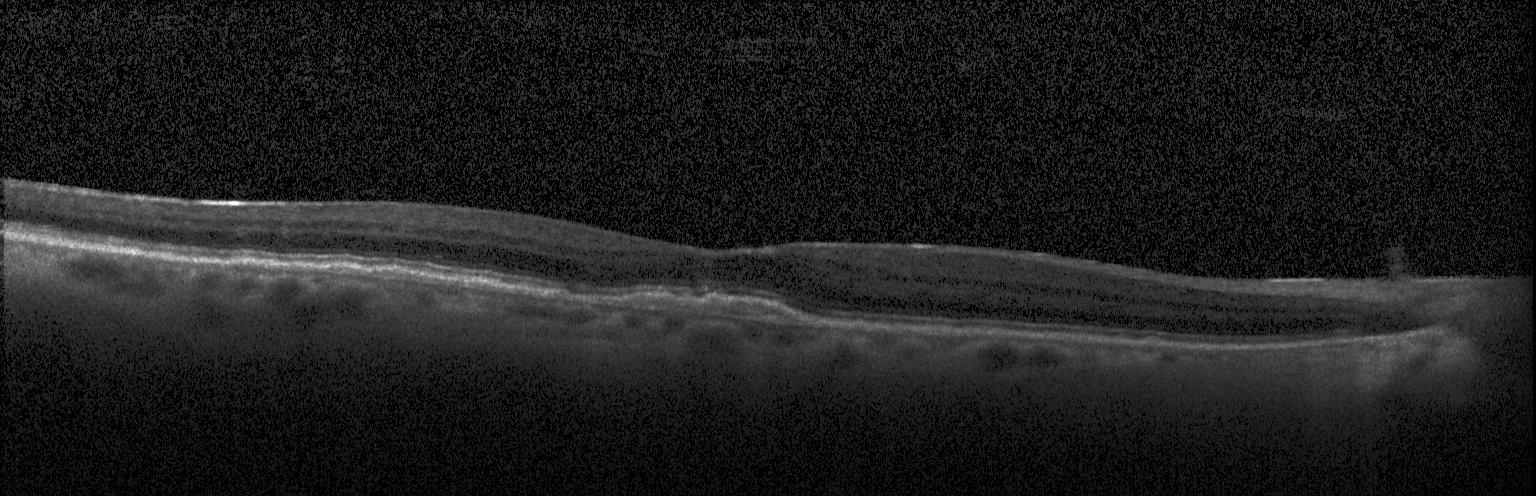

Optical coherence tomography scan, spectral-domain OCT. Assessment: choroidal neovascularization (CNV).